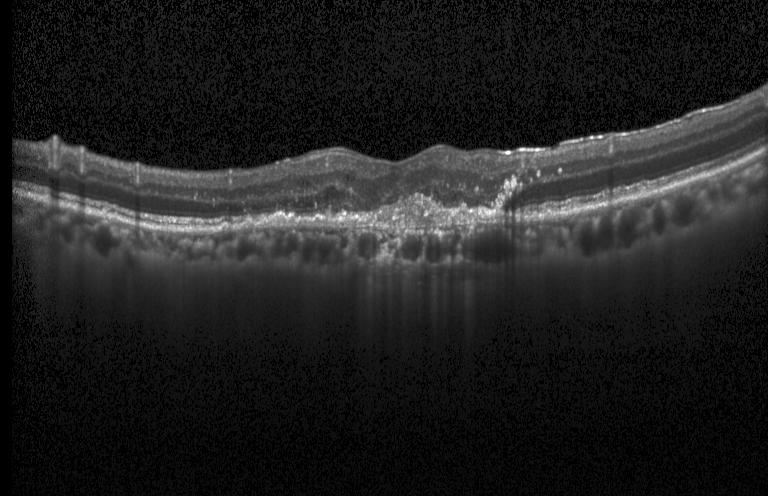 Through the macula, retinal OCT B-scan — Diagnosis: a choroidal neovascular membrane.